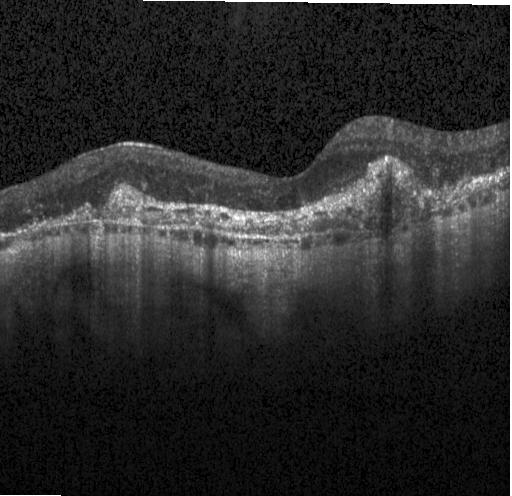
Retinal OCT B-scan; acquired on a Heidelberg Spectralis — Dx: choroidal neovascularization.